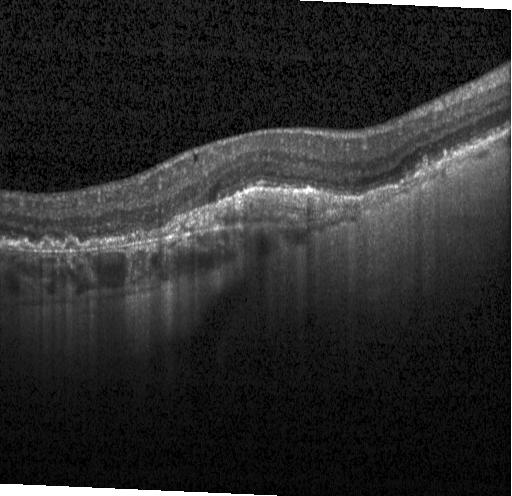 Finding: choroidal neovascularization.